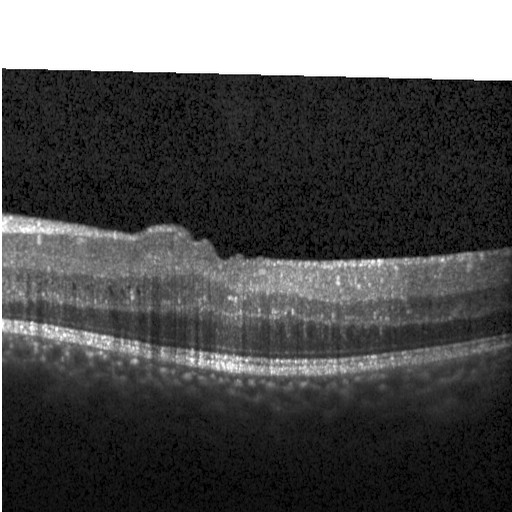
Retinal OCT cross-section; acquired on a Heidelberg Spectralis.
OCT finding: DME.